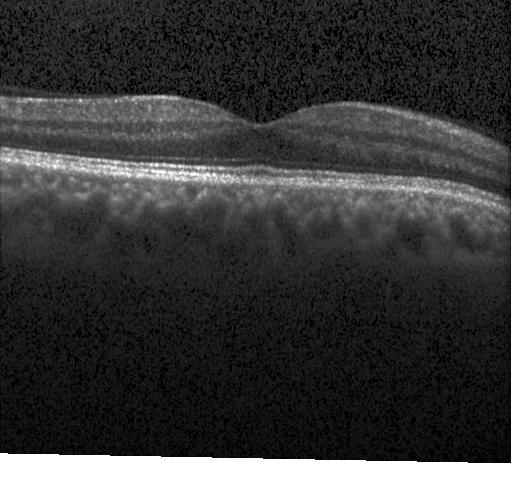

OCT scan showing neither choroidal neovascularization, diabetic macular edema, nor drusen.